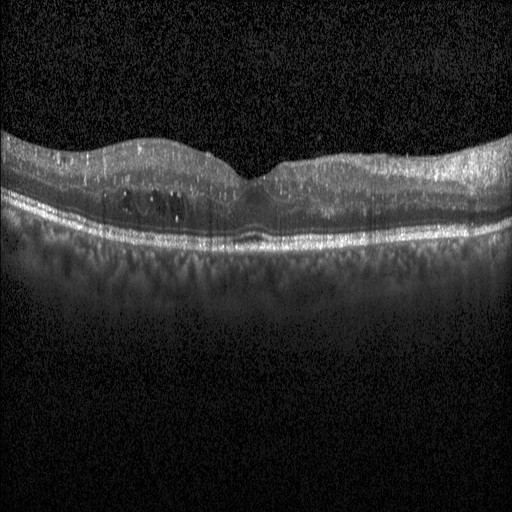 Spectral-domain OCT. Optical coherence tomography B-scan
The scan shows diabetic macular edema.